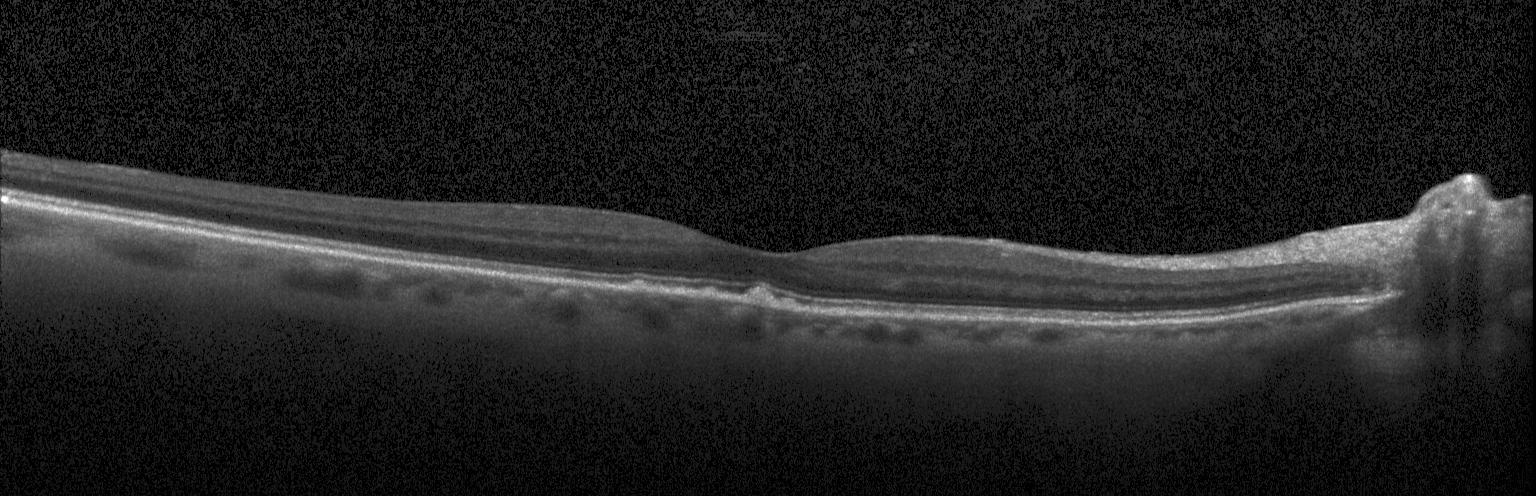
Diagnosis: drusen.